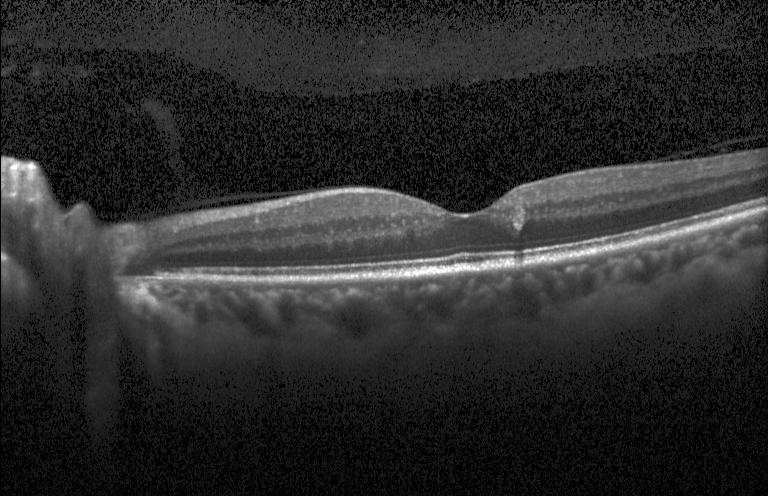

OCT B-scan
The scan shows no choroidal neovascularization, no diabetic macular edema, and no drusen.